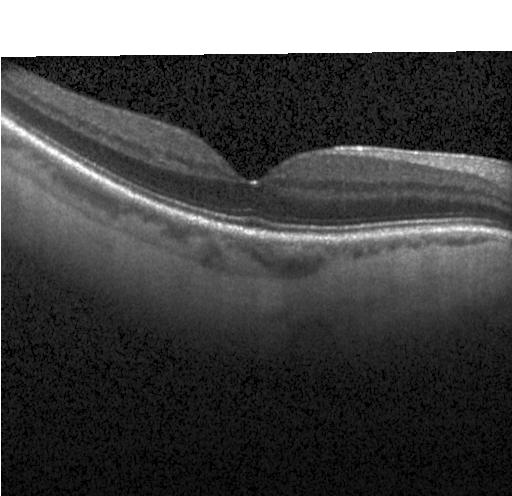 OCT line scan, SD-OCT, through the macula — The scan shows no CNV, DME, or drusen.